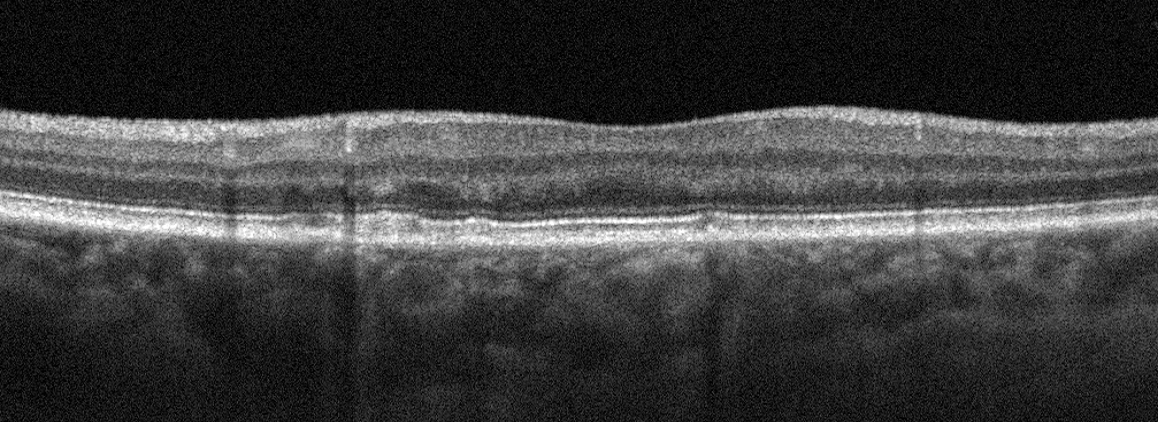 Oculus sinister; Optovue Avanti RTVue XR; optical coherence tomography scan; macular scan — Age-related macular degeneration.